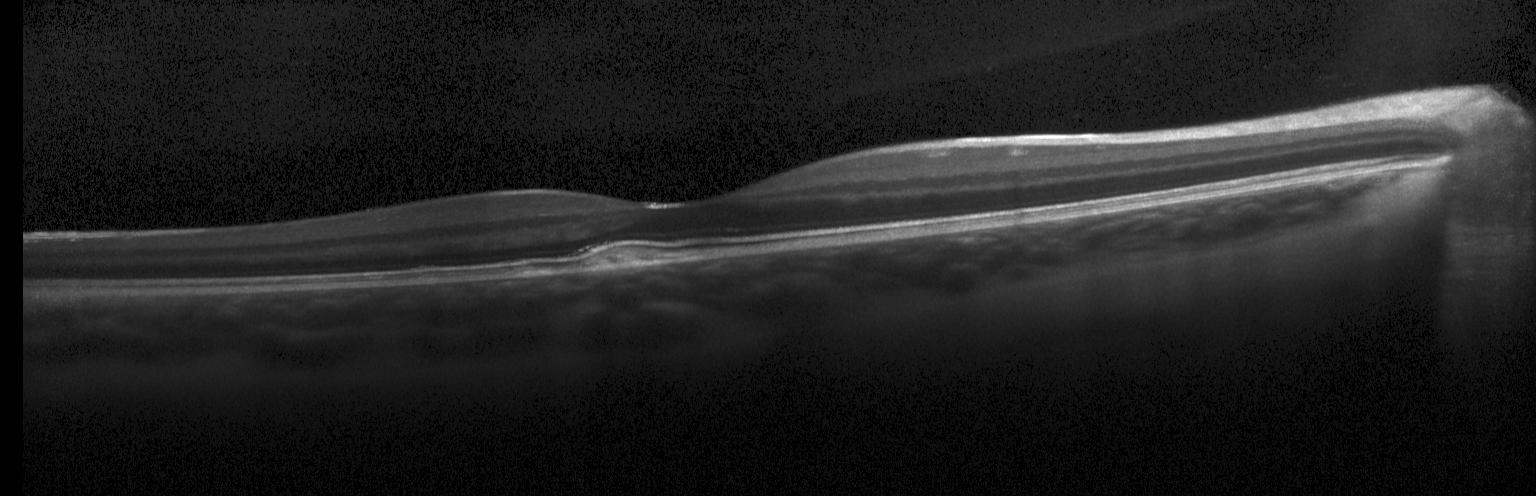 Optical coherence tomography B-scan
The scan shows drusen.